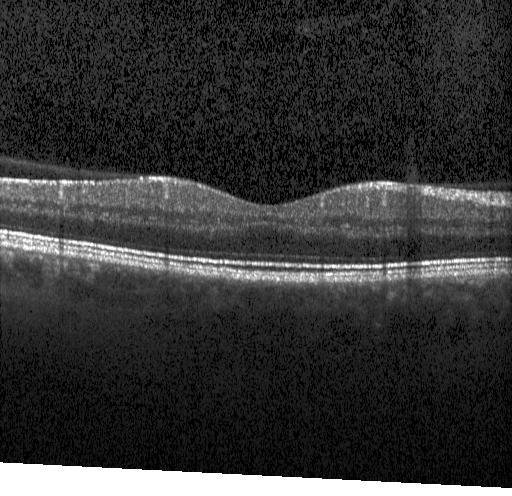 Retinal OCT cross-section; SD-OCT; horizontal scan through the fovea.
Impression: no choroidal neovascularization, diabetic macular edema, or drusen.